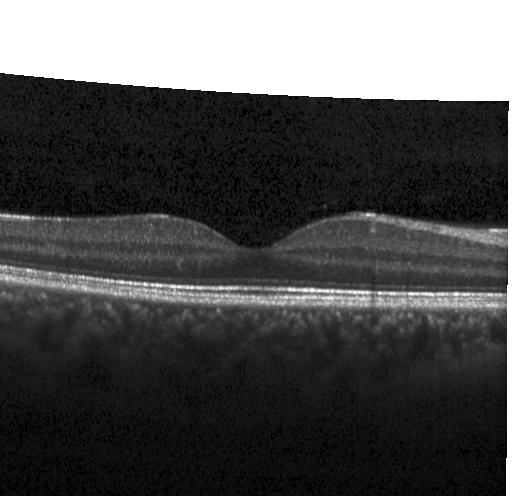

Impression: no choroidal neovascularization, diabetic macular edema, or drusen.